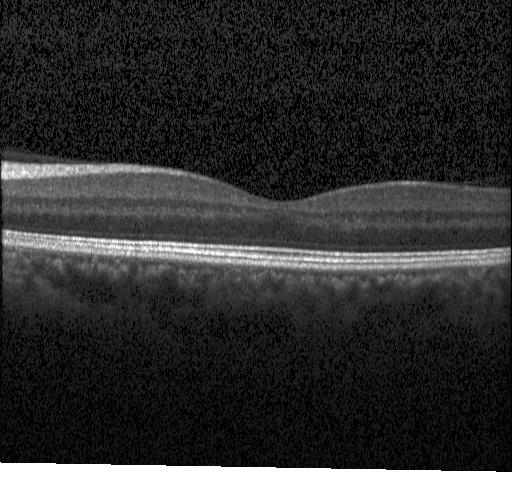 Retinal OCT B-scan
Impression: neither choroidal neovascularization, diabetic macular edema, nor drusen.